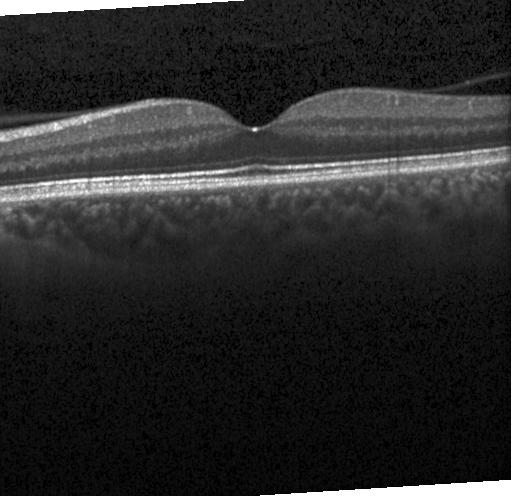 Spectral-domain OCT. OCT B-scan — Finding: neither choroidal neovascularization, diabetic macular edema, nor drusen.